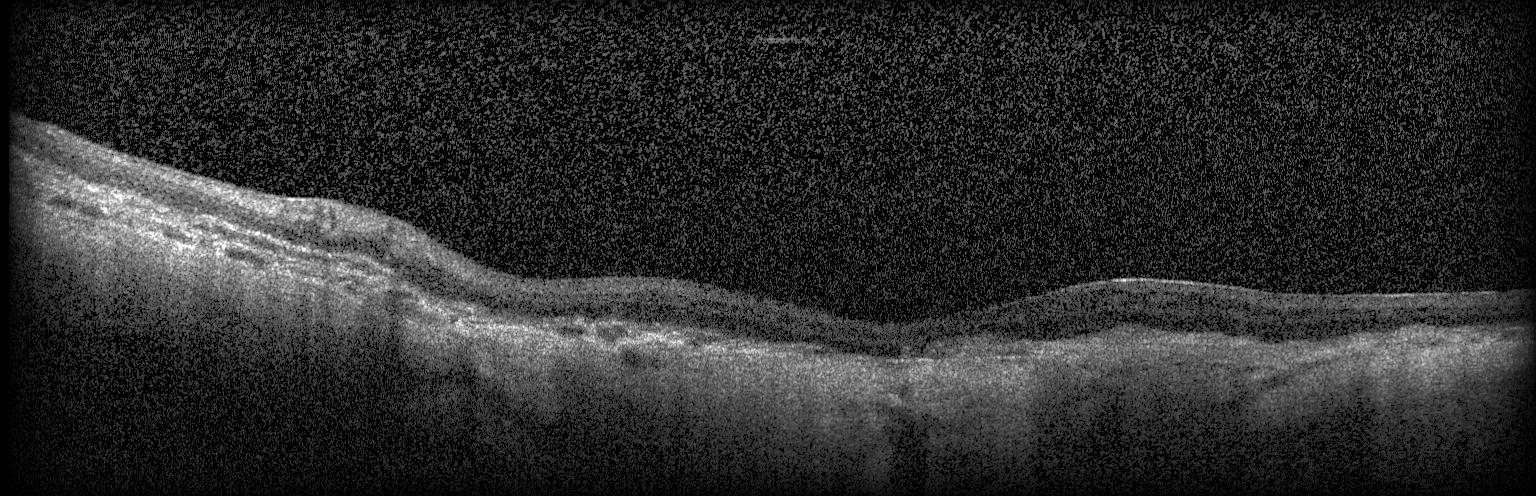
OCT finding: a choroidal neovascular membrane.